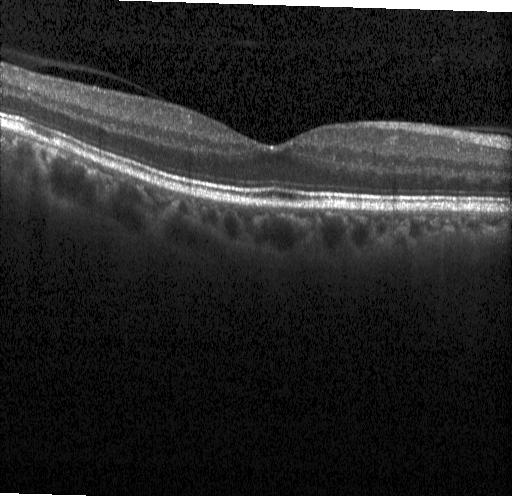
Macular OCT: no CNV, DME, or drusen.